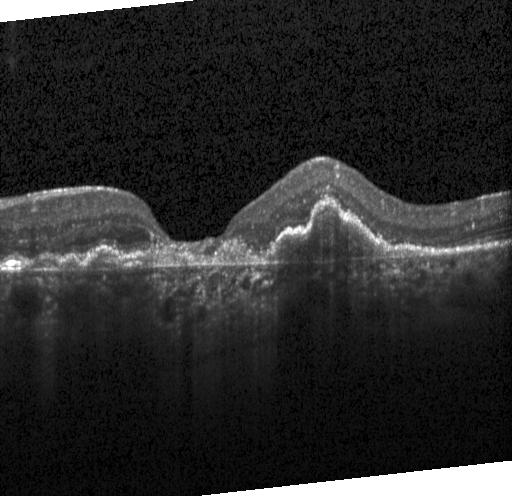

Diagnosis: a choroidal neovascular membrane.